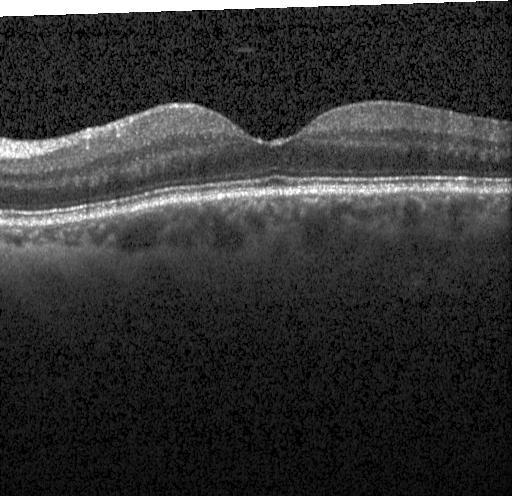 Spectral-domain OCT B-scan: no choroidal neovascularization, diabetic macular edema, or drusen.